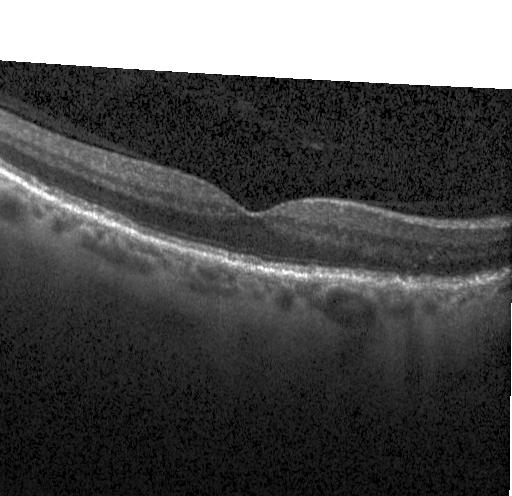
Spectral-domain optical coherence tomography; retinal OCT cross-section.
Impression: no evidence of choroidal neovascularization, diabetic macular edema, or drusen.